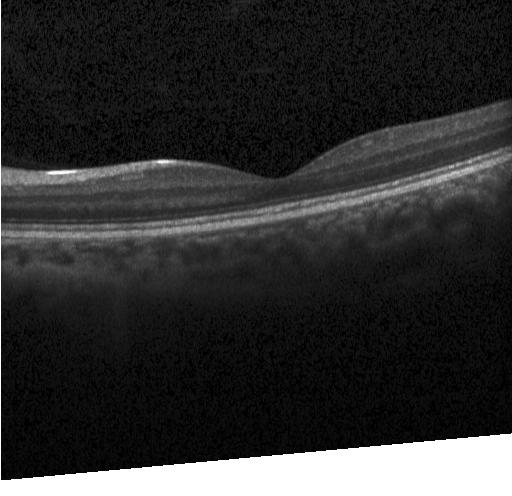

SD-OCT; Heidelberg Spectralis; through the macula; OCT line scan.
Diagnosis: no choroidal neovascularization, no diabetic macular edema, and no drusen.